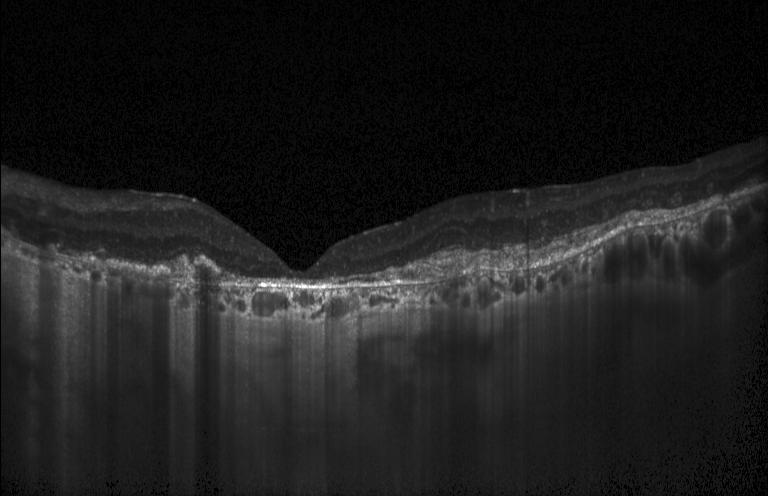
SD-OCT · OCT B-scan · Heidelberg Spectralis OCT system · through the macula. Dx: a choroidal neovascular membrane.